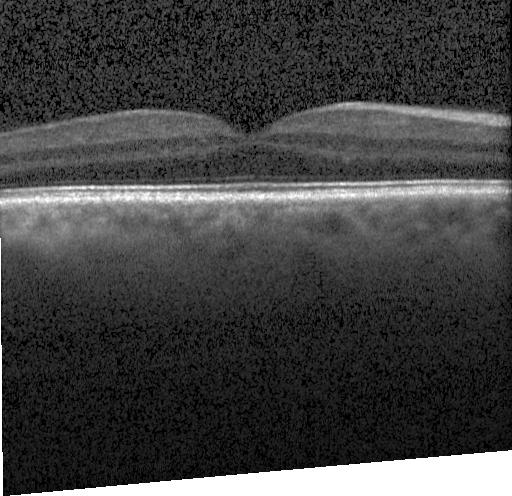
Spectral-domain OCT · OCT B-scan.
This B-scan demonstrates neither choroidal neovascularization, diabetic macular edema, nor drusen.